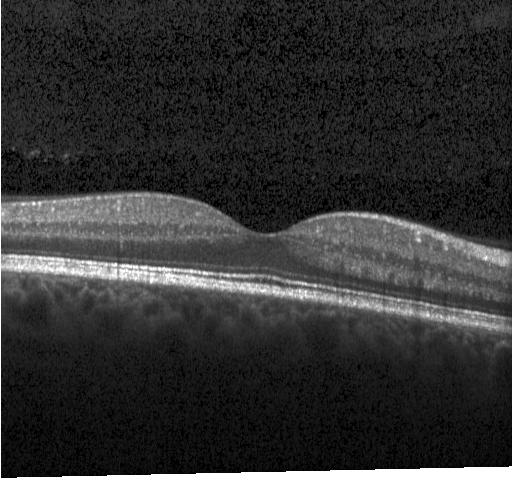
Diagnosis: no CNV, DME, or drusen.